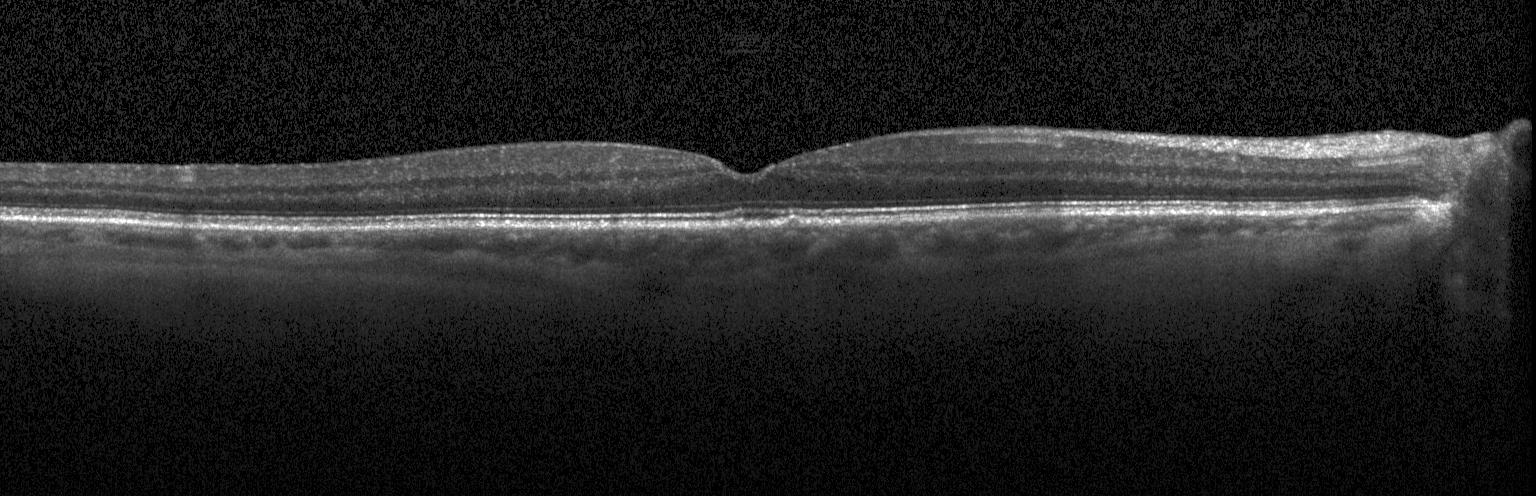 SD-OCT · horizontal scan through the fovea · optical coherence tomography B-scan
Diagnosis: sub-RPE drusenoid deposits.